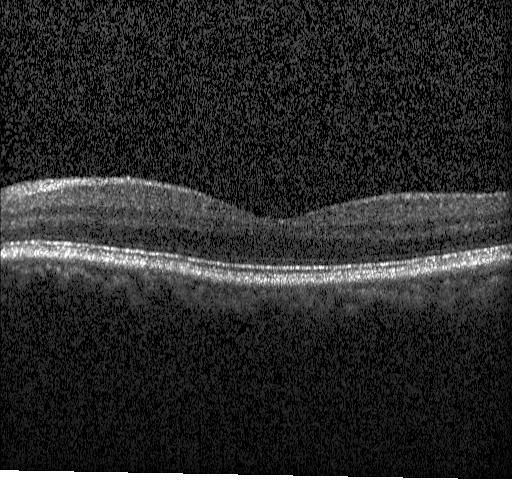 Impression: no evidence of choroidal neovascularization, diabetic macular edema, or drusen.